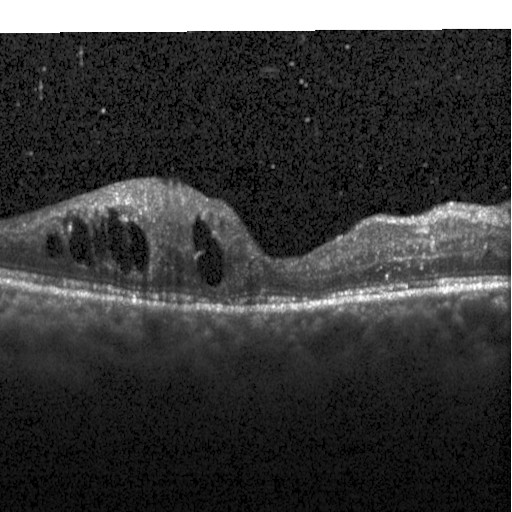 Retinal OCT B-scan. Impression: DME.